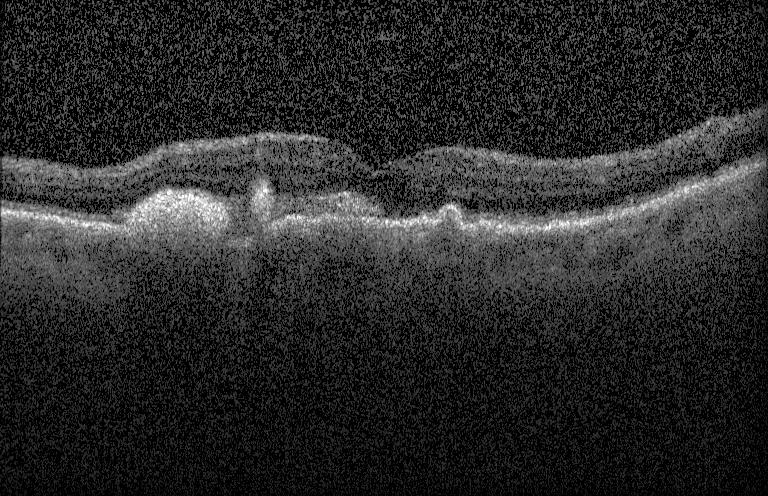

Impression: a choroidal neovascular membrane.